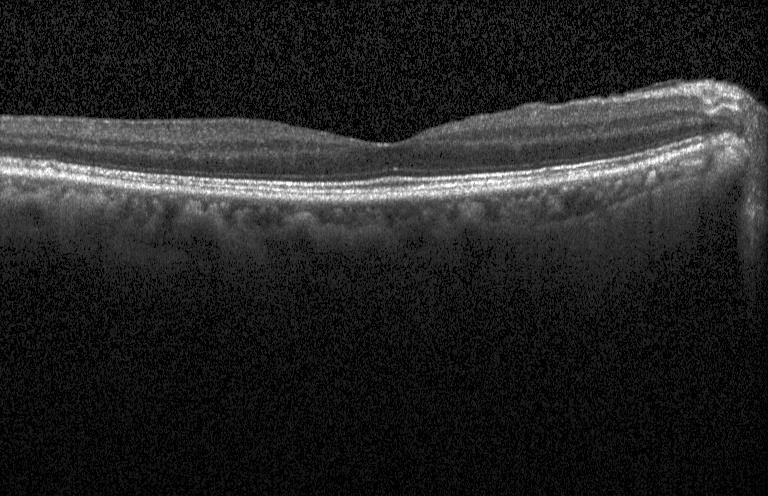
Assessment: no choroidal neovascularization, no diabetic macular edema, and no drusen.